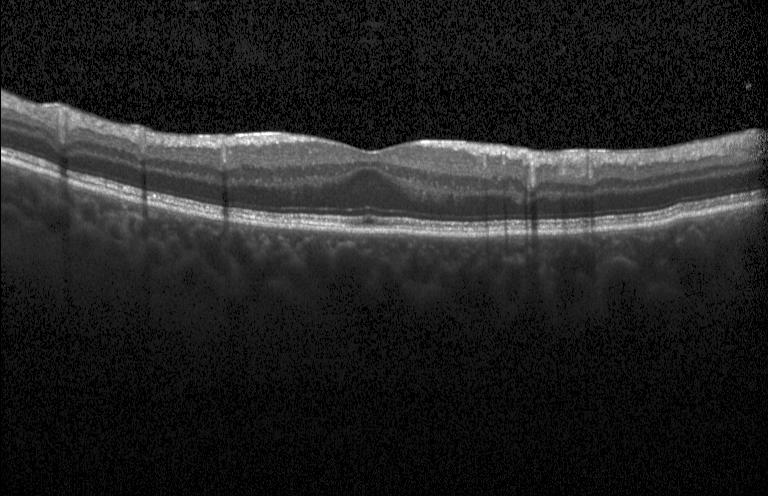 Retinal OCT B-scan.
Impression: no CNV, no DME, and no drusen.